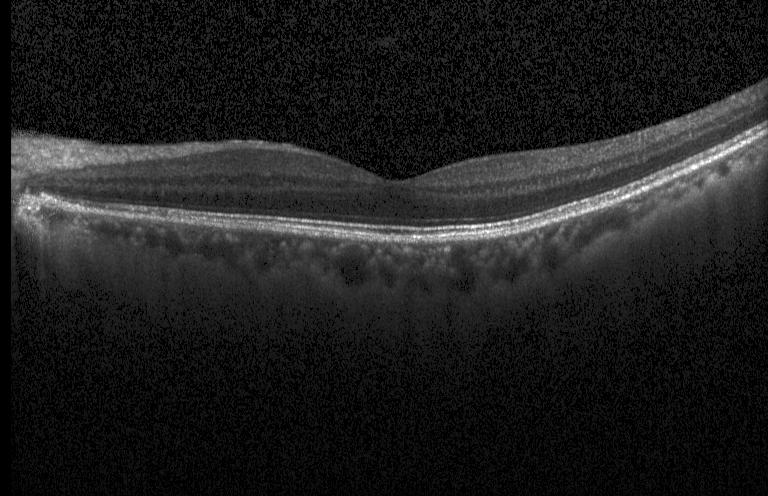 Assessment: no evidence of CNV, DME, or drusen.